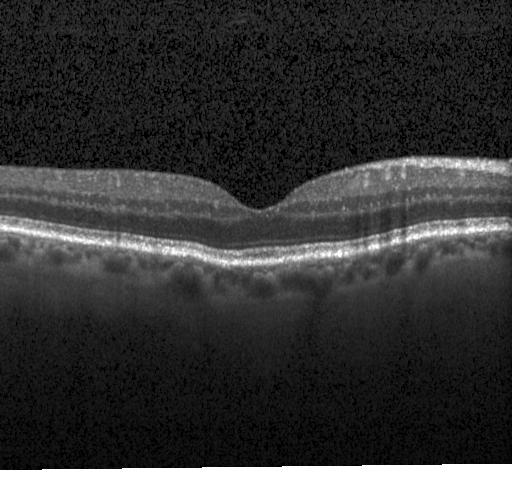
Retinal OCT cross-section showing no choroidal neovascularization, diabetic macular edema, or drusen.